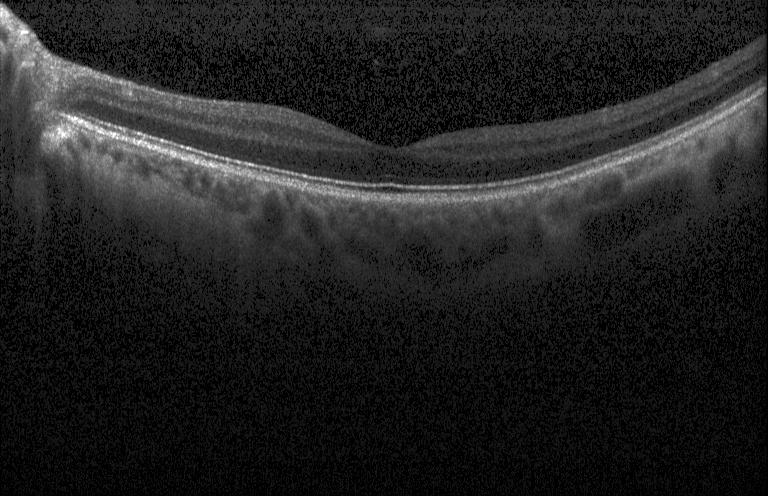 Optical coherence tomography B-scan; acquired on a Heidelberg Spectralis. Diagnosis: no choroidal neovascularization, no diabetic macular edema, and no drusen.